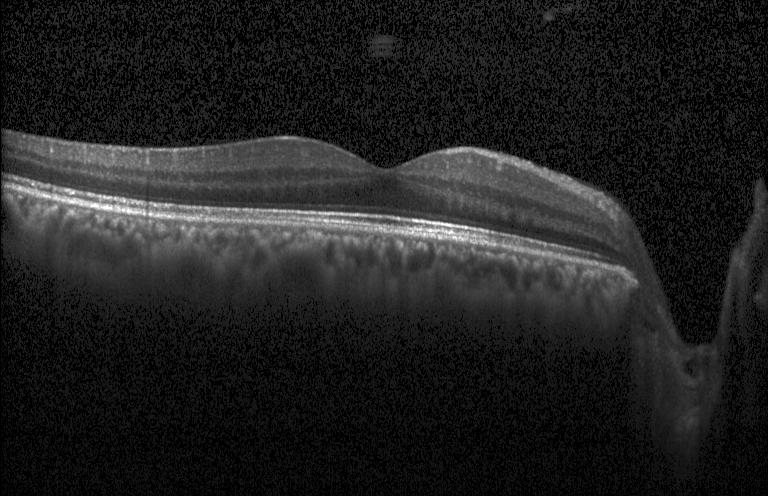
Retinal OCT cross-section; Heidelberg Spectralis.
This B-scan demonstrates neither choroidal neovascularization, diabetic macular edema, nor drusen.